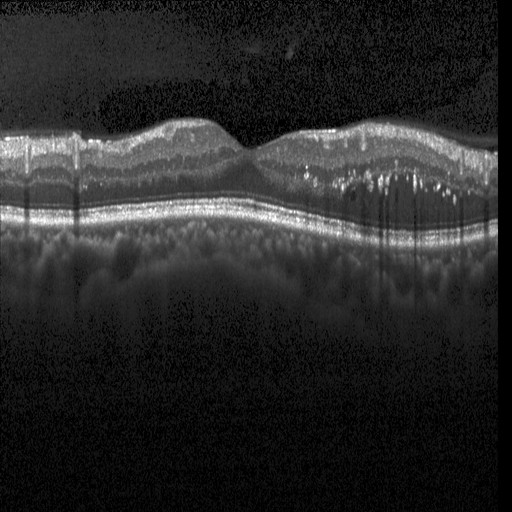
SD-OCT · OCT B-scan · macular scan.
Diagnosis: diabetic macular edema (DME).